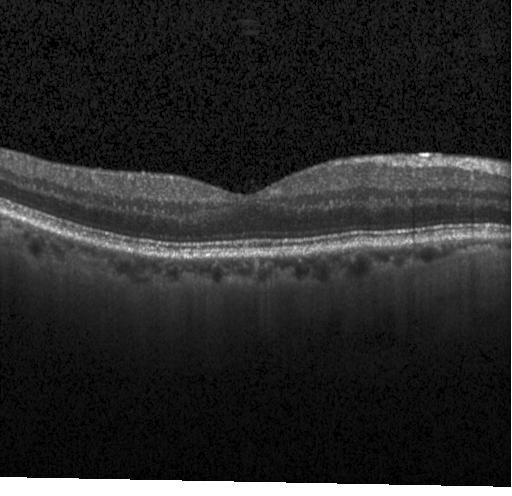
Retinal OCT B-scan; centered on the fovea; instrument: Heidelberg Spectralis; SD-OCT — Finding: no choroidal neovascularization, no diabetic macular edema, and no drusen.